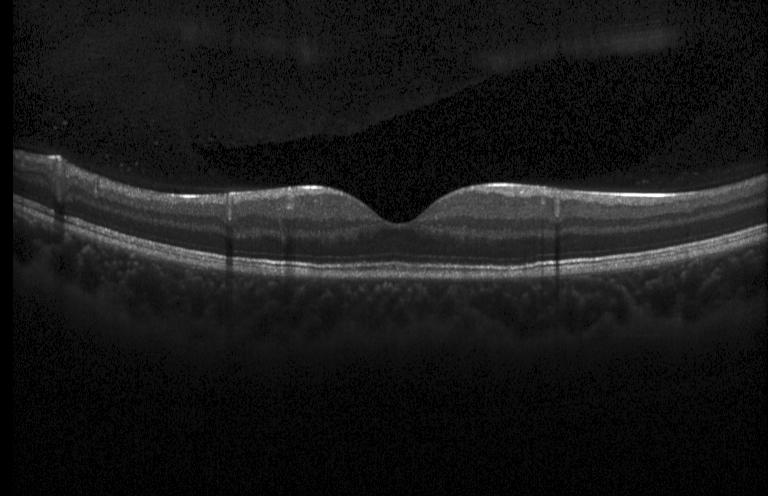

OCT B-scan, through the macula
Finding: no evidence of choroidal neovascularization, diabetic macular edema, or drusen.